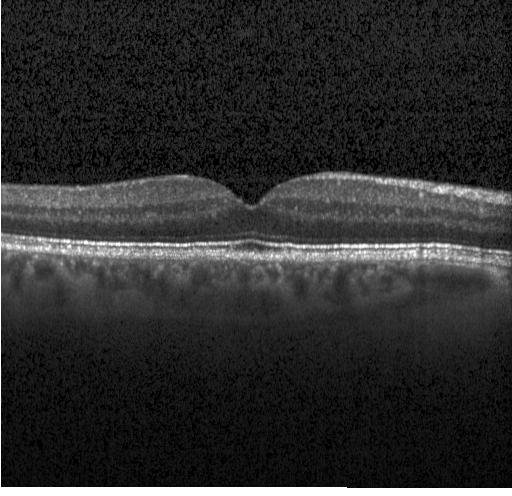 Fovea-centered; retinal OCT cross-section; spectral-domain optical coherence tomography; acquired on a Heidelberg Spectralis.
This B-scan demonstrates no choroidal neovascularization, no diabetic macular edema, and no drusen.